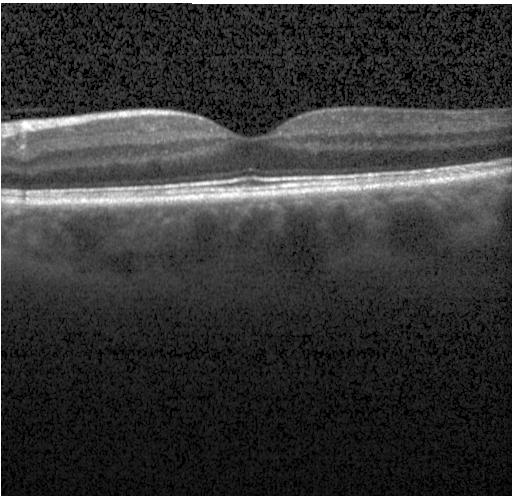
Instrument: Heidelberg Spectralis. OCT line scan. Fovea-centered
Neither choroidal neovascularization, diabetic macular edema, nor drusen.